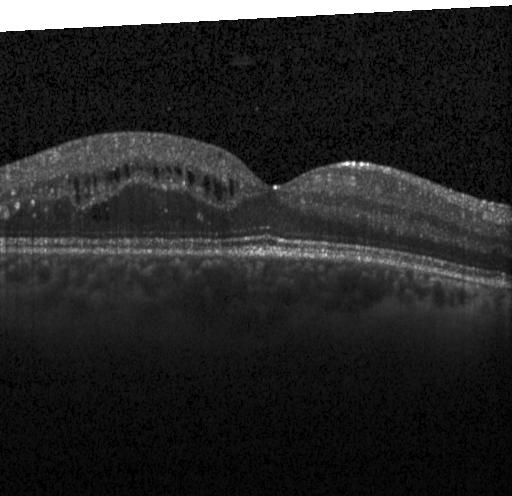
Retinal OCT B-scan. Horizontal scan through the fovea.
Impression: diabetic macular edema.